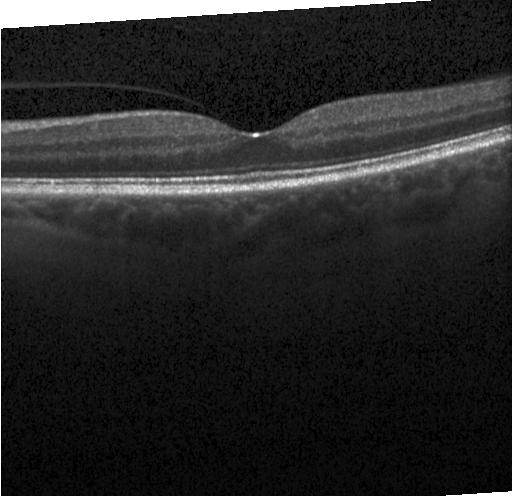

The scan shows no choroidal neovascularization, no diabetic macular edema, and no drusen.